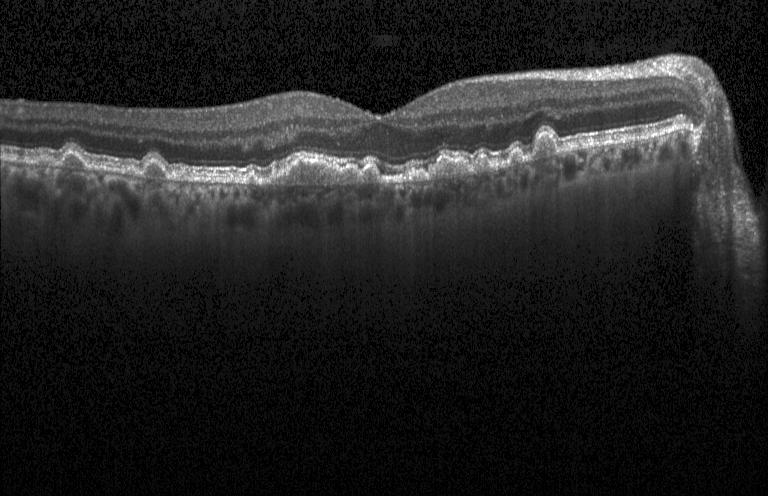

OCT line scan. Macular scan. Heidelberg Spectralis OCT system
The scan shows multiple drusen.